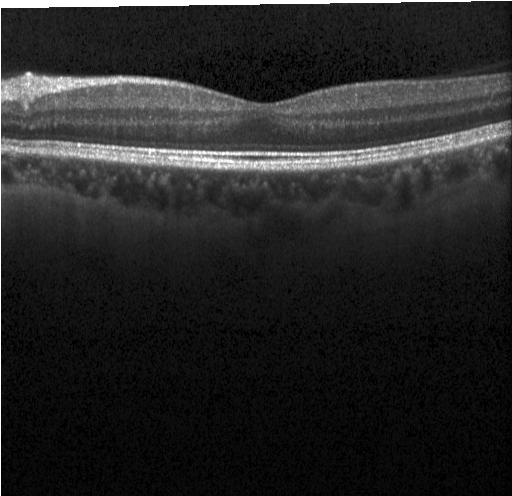

Spectral-domain optical coherence tomography; optical coherence tomography B-scan; Heidelberg Spectralis
Macular OCT: no choroidal neovascularization, no diabetic macular edema, and no drusen.